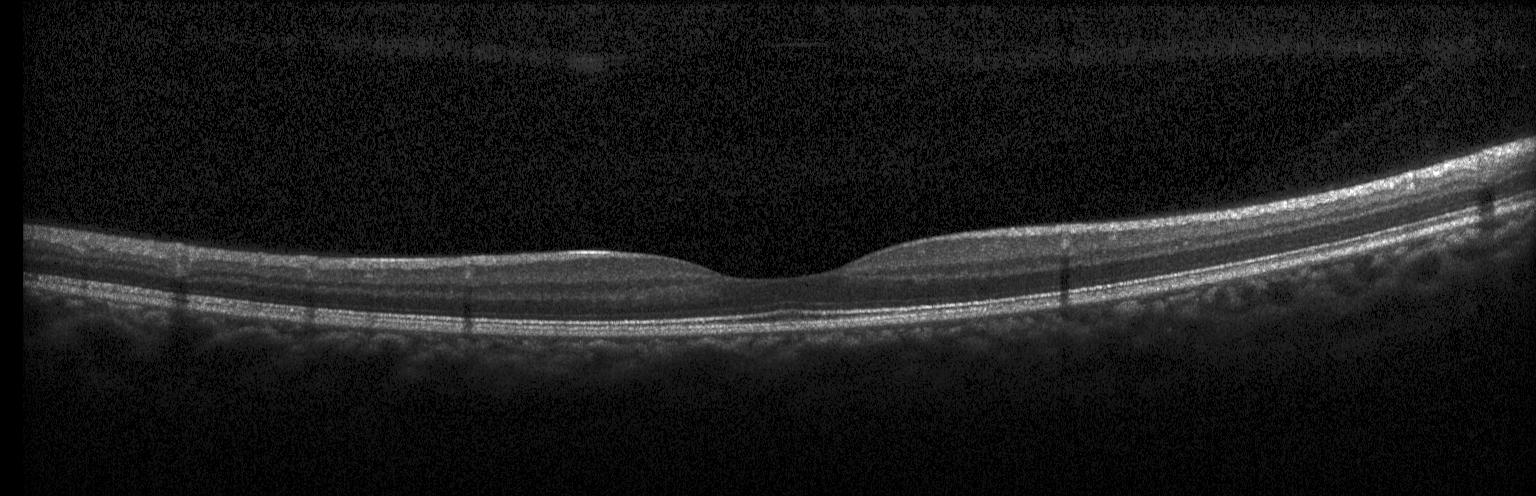 Heidelberg Spectralis OCT system. Spectral-domain optical coherence tomography. OCT line scan. Horizontal scan through the fovea.
Assessment: no CNV, DME, or drusen.